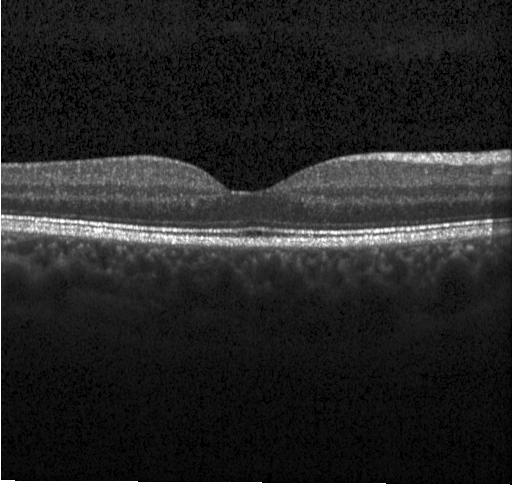 Impression: no choroidal neovascularization, no diabetic macular edema, and no drusen.